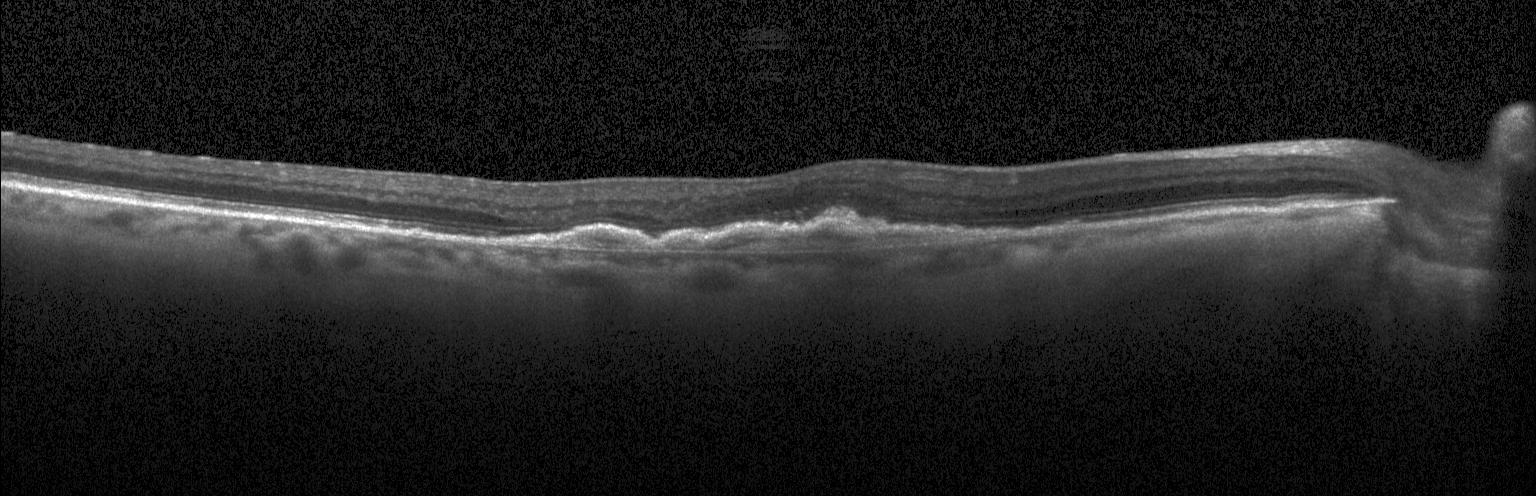 Spectral-domain OCT B-scan: a choroidal neovascular membrane.